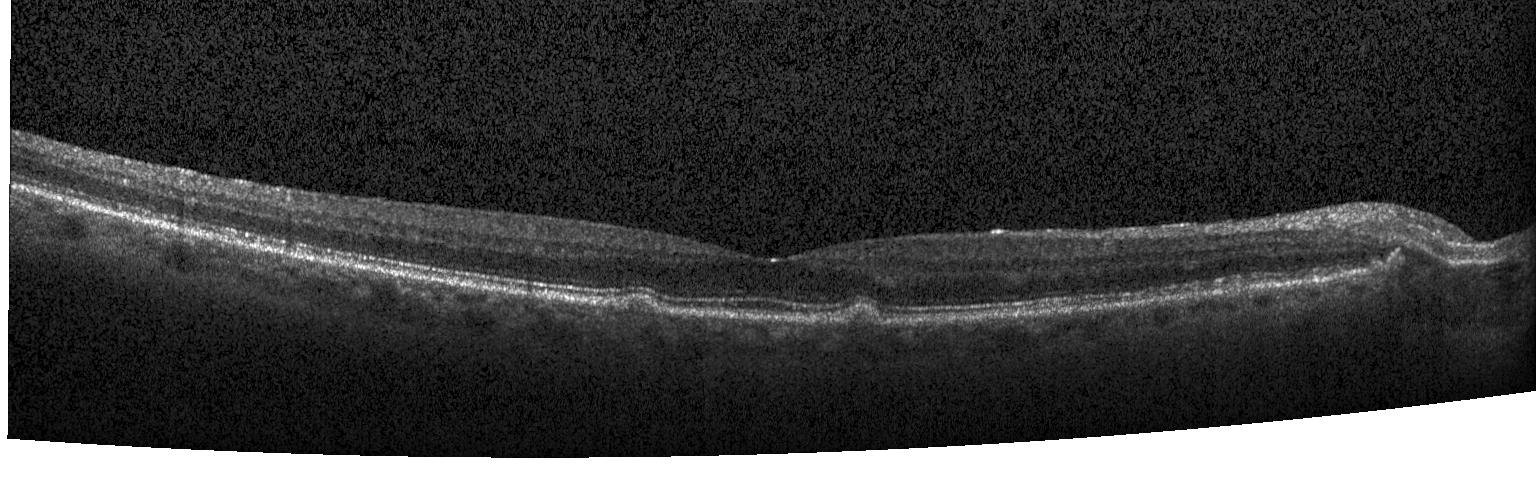 Finding: sub-RPE drusenoid deposits.